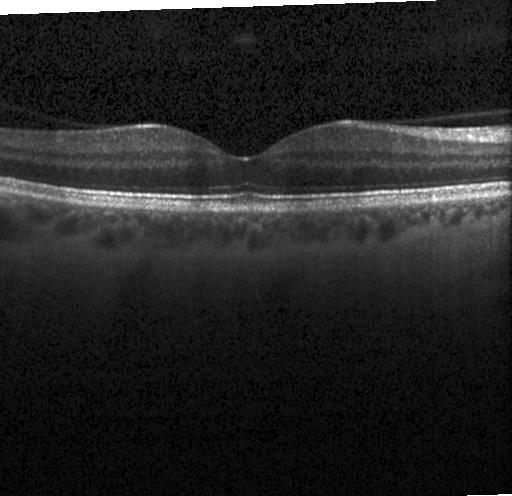

Spectral-domain OCT; OCT line scan; Heidelberg Spectralis
Assessment: neither CNV, DME, nor drusen.